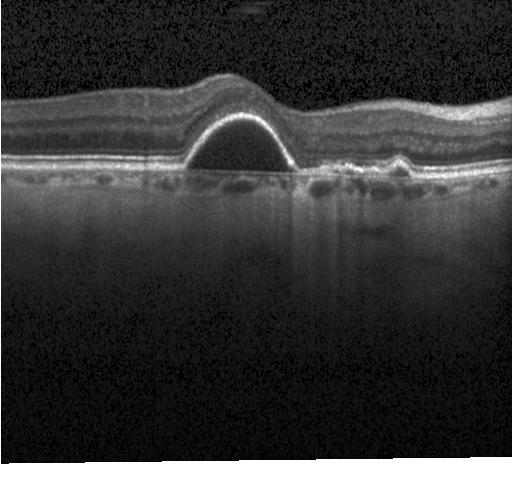
Heidelberg Spectralis; retinal OCT cross-section; SD-OCT; through the macula — Diagnosis: choroidal neovascularization.